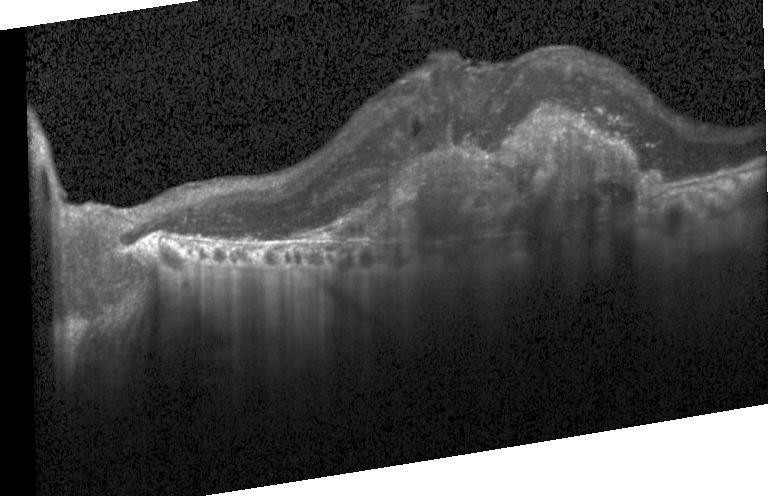

OCT B-scan, Heidelberg Spectralis, SD-OCT. The scan shows a choroidal neovascular membrane.